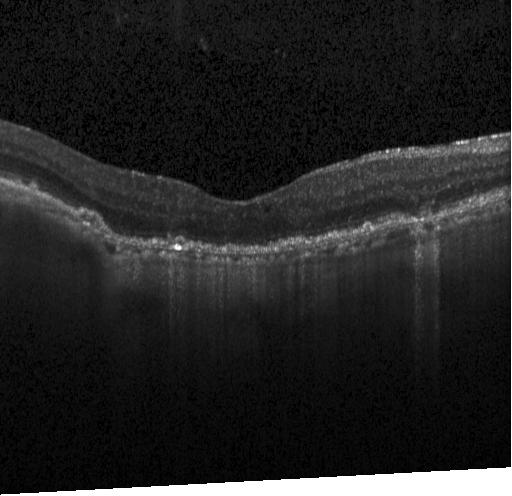 Optical coherence tomography B-scan. Spectral-domain optical coherence tomography — Diagnosis: CNV.